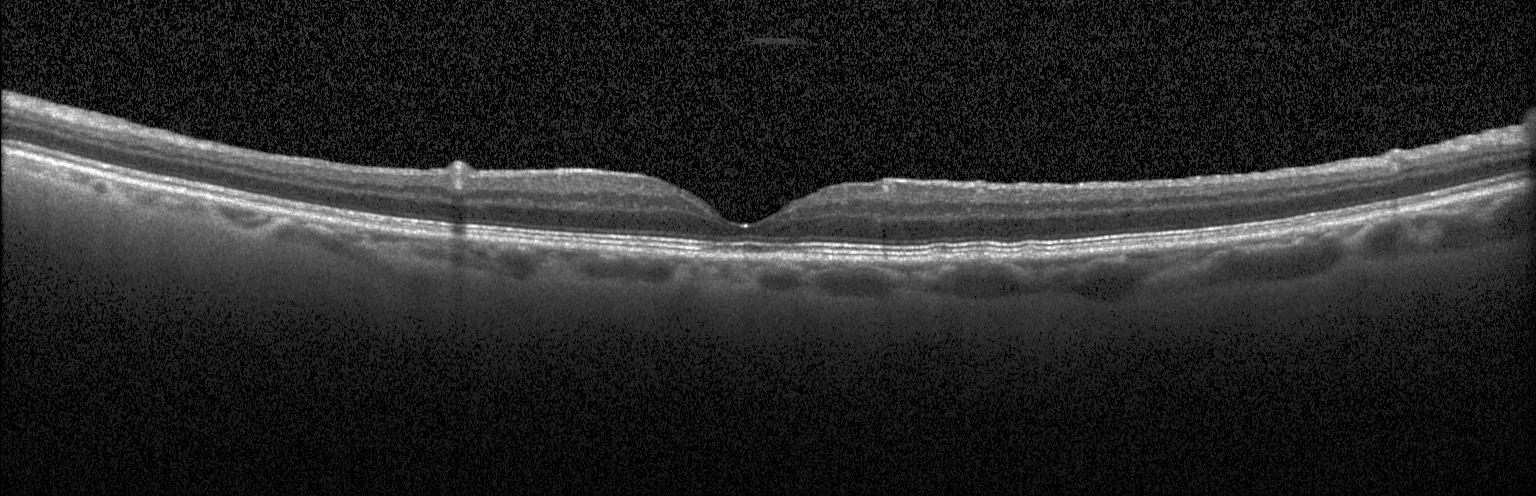
Optical coherence tomography B-scan.
No evidence of choroidal neovascularization, diabetic macular edema, or drusen.